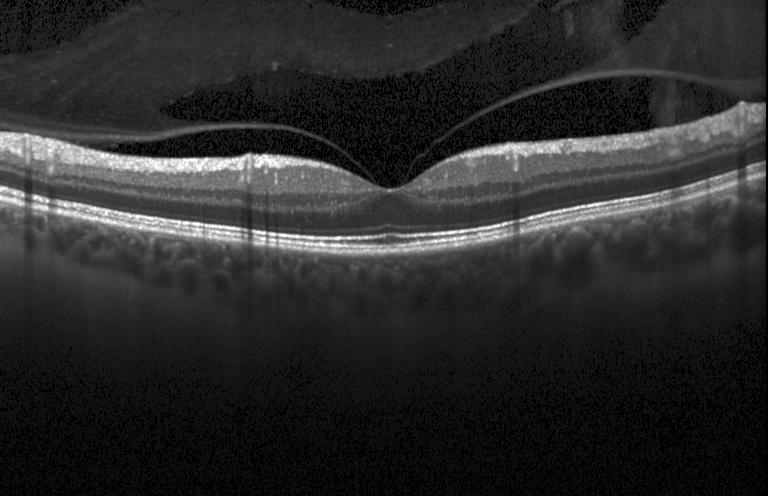
OCT line scan; SD-OCT
No choroidal neovascularization, no diabetic macular edema, and no drusen.